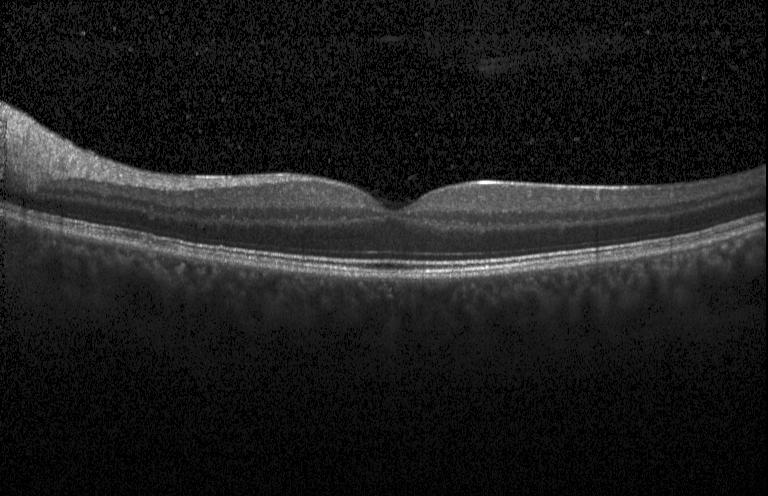 Dx: no choroidal neovascularization, diabetic macular edema, or drusen.